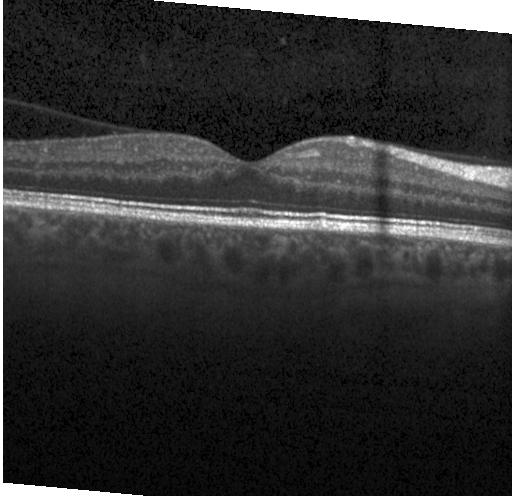 Impression: no choroidal neovascularization, no diabetic macular edema, and no drusen.